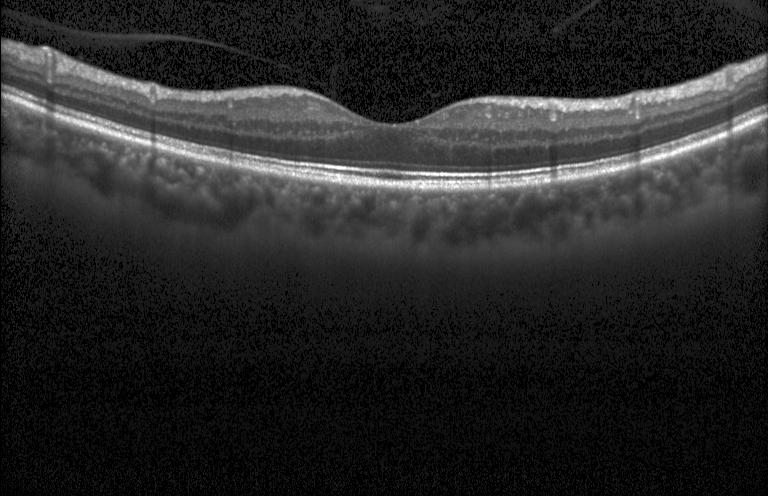

OCT finding: no choroidal neovascularization, diabetic macular edema, or drusen.